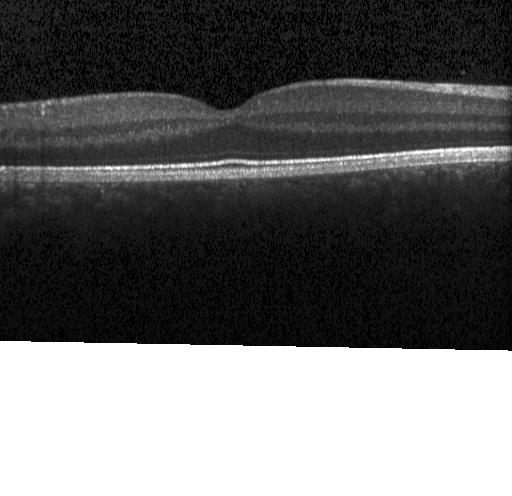
The scan shows neither CNV, DME, nor drusen.